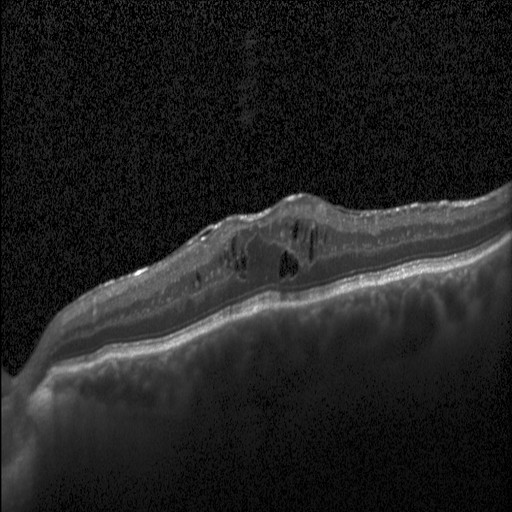

Macular OCT demonstrating diabetic macular edema (DME).